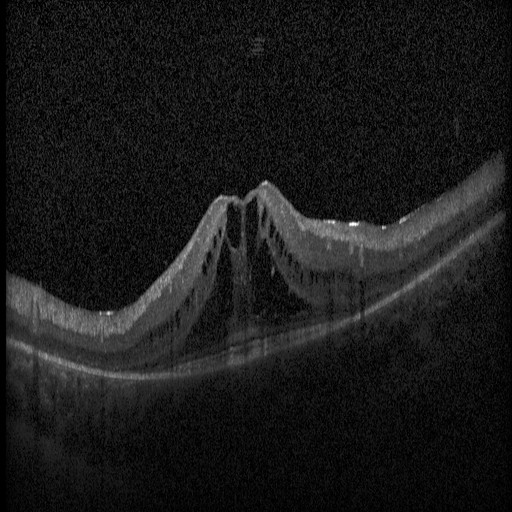
OCT line scan — Finding: diabetic macular edema.